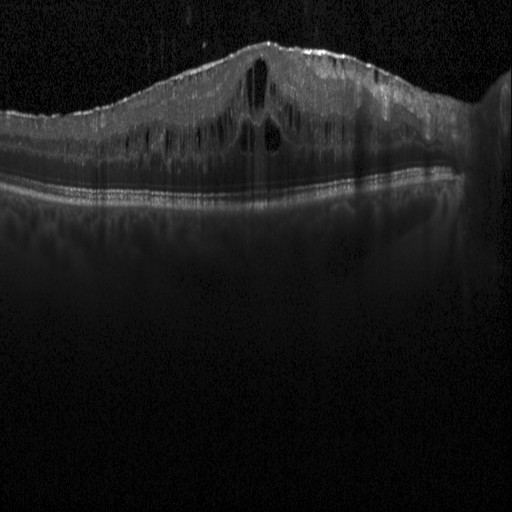

Retinal OCT B-scan. OCT finding: diabetic macular edema (DME).